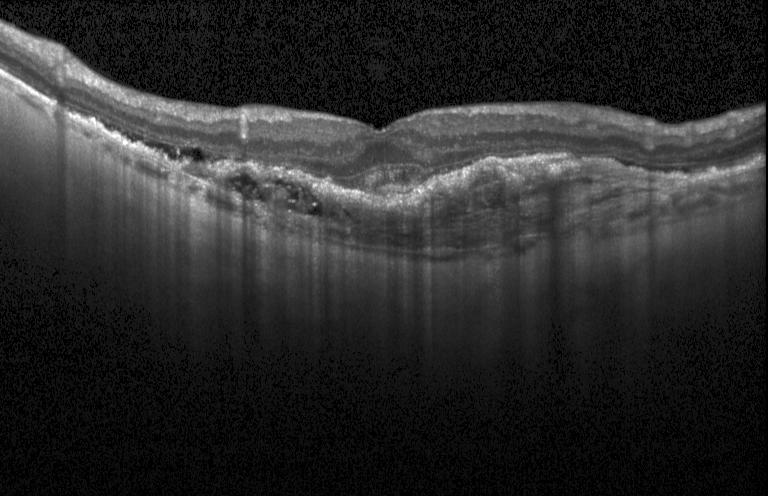 Finding: CNV.